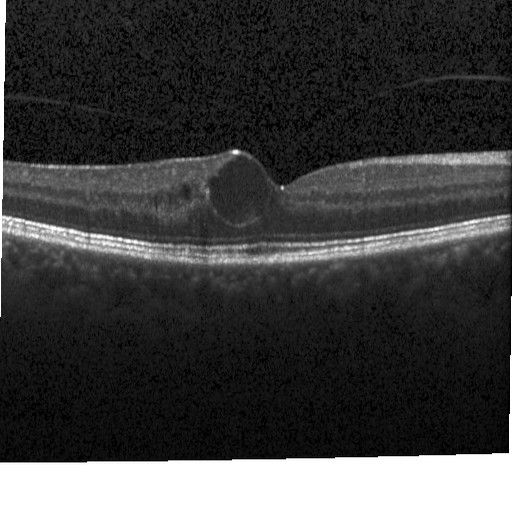

SD-OCT. Heidelberg Spectralis OCT system. OCT line scan. Through the macula. Macular OCT: DME.